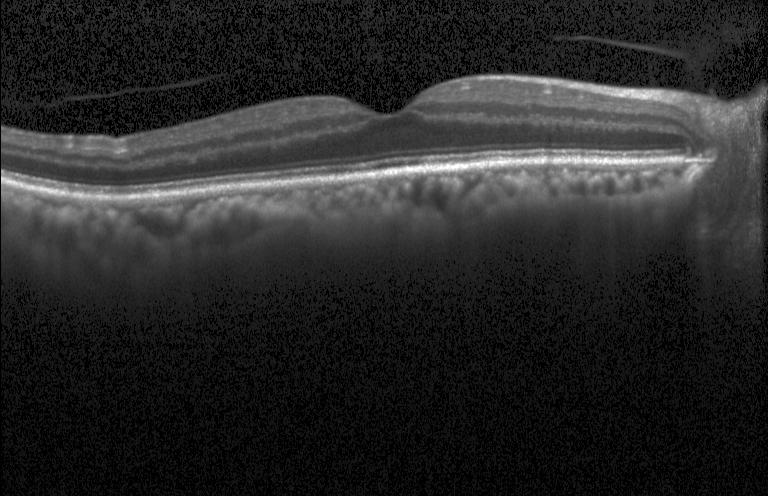

OCT line scan — Impression: no choroidal neovascularization, diabetic macular edema, or drusen.